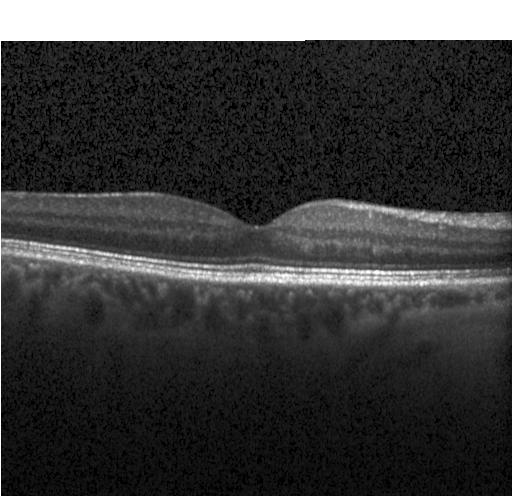
No choroidal neovascularization, no diabetic macular edema, and no drusen.